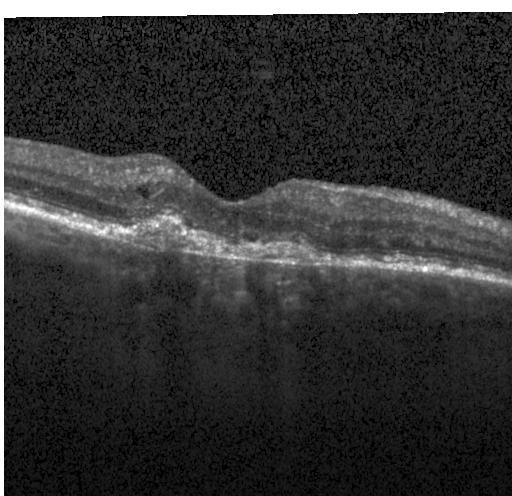
Spectral-domain OCT · retinal OCT B-scan · centered on the fovea — Diagnosis: a choroidal neovascular membrane.